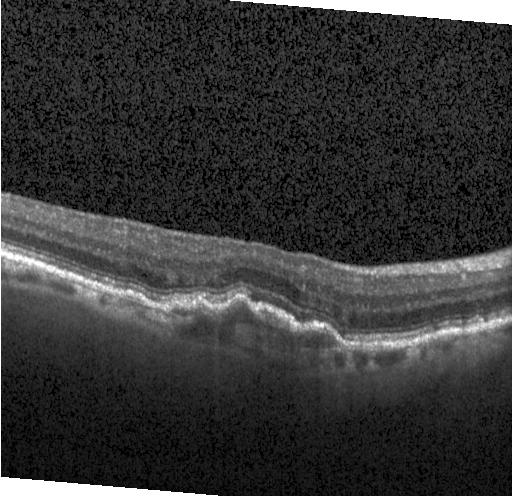 OCT line scan. Diagnosis: choroidal neovascularization.